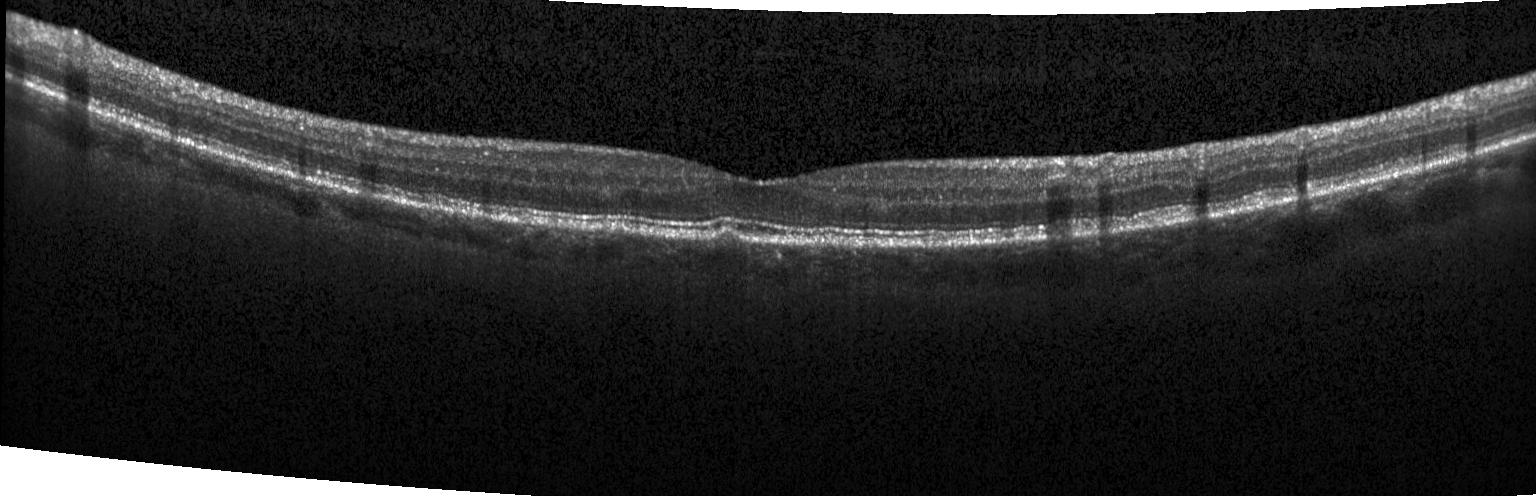 Finding: multiple drusen.